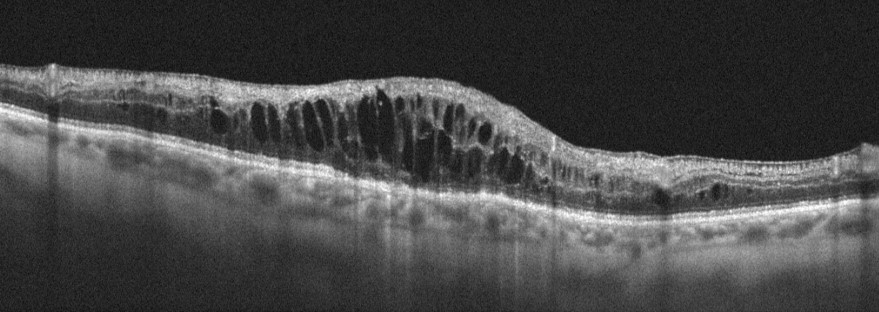

OCT line scan, instrument: Optovue Avanti RTVue XR
Dx: diabetic macular edema.